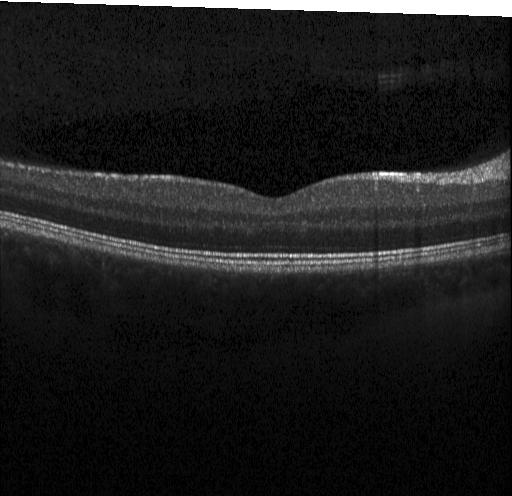
Assessment: no choroidal neovascularization, diabetic macular edema, or drusen.